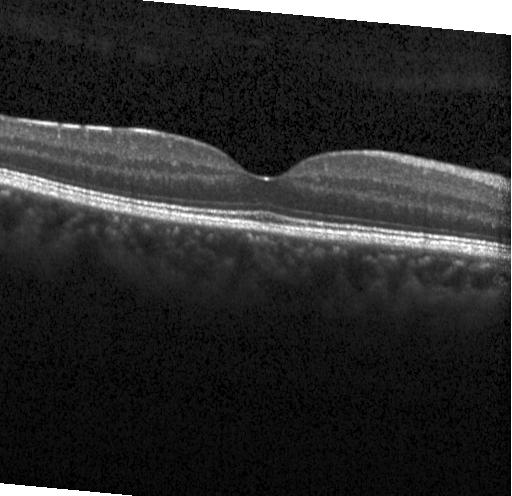
Macular OCT: no CNV, DME, or drusen.